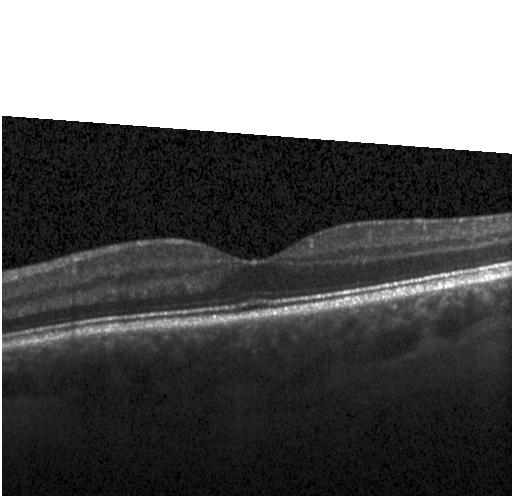
Optical coherence tomography B-scan · acquired on a Heidelberg Spectralis. Assessment: no CNV, no DME, and no drusen.